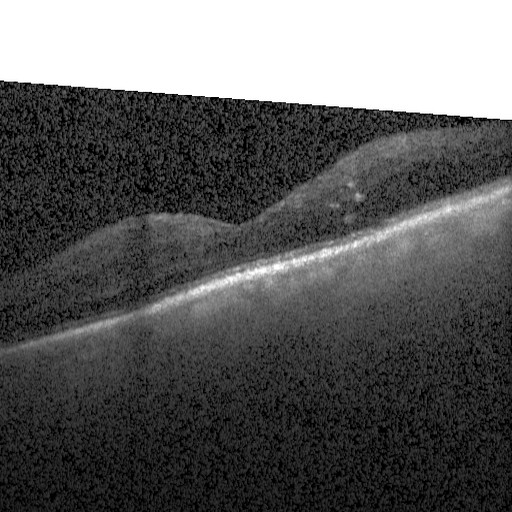
Finding: diabetic macular edema (DME).